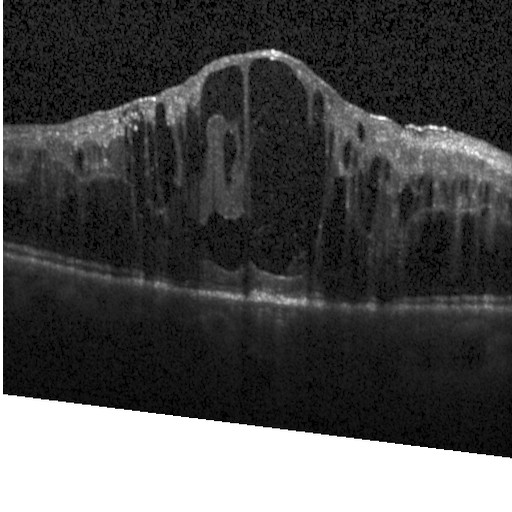

Through the macula · spectral-domain OCT · OCT line scan · instrument: Heidelberg Spectralis. Impression: diabetic macular edema (DME).